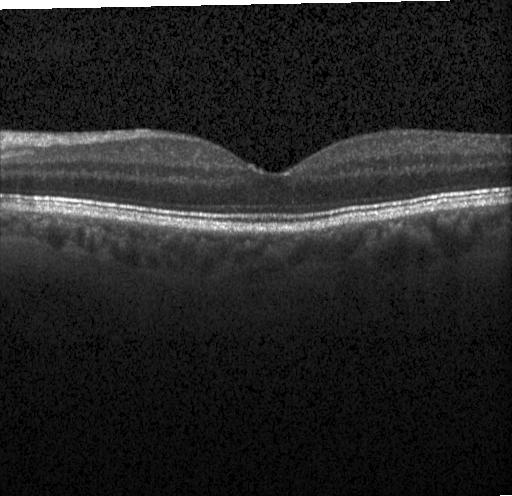
Optical coherence tomography B-scan — Impression: no CNV, no DME, and no drusen.